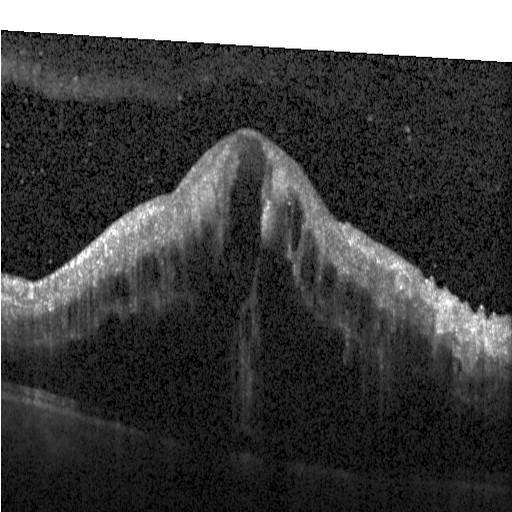

OCT line scan — Impression: diabetic macular edema.